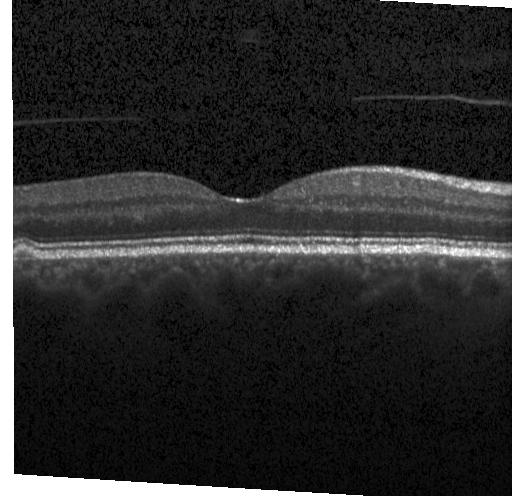 Diagnosis: drusen.